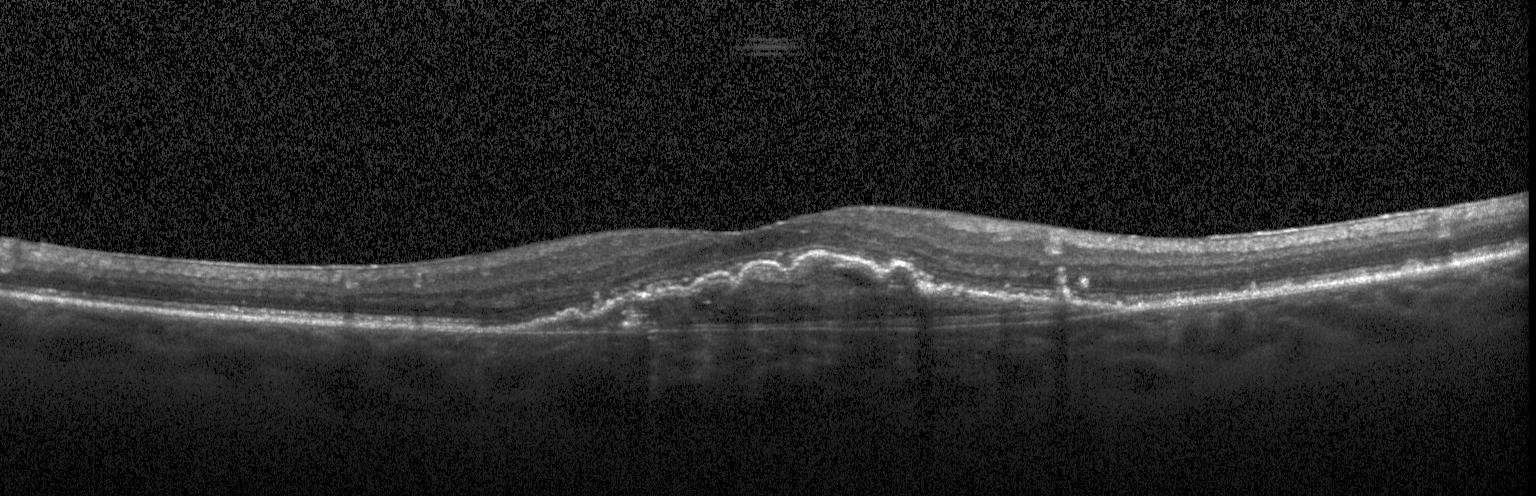 Macular OCT demonstrating a choroidal neovascular membrane.